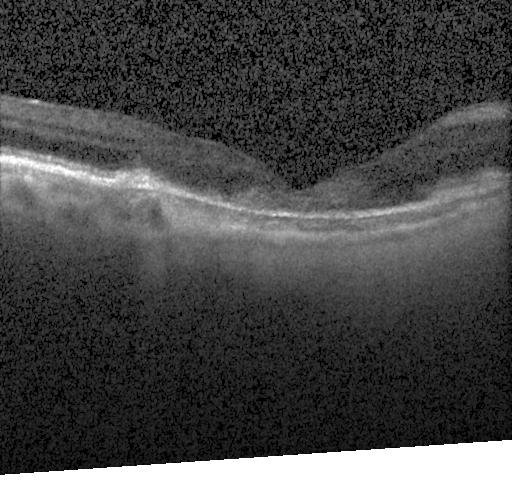 Centered on the fovea · spectral-domain optical coherence tomography · optical coherence tomography scan · Heidelberg Spectralis — OCT finding: choroidal neovascularization (CNV).